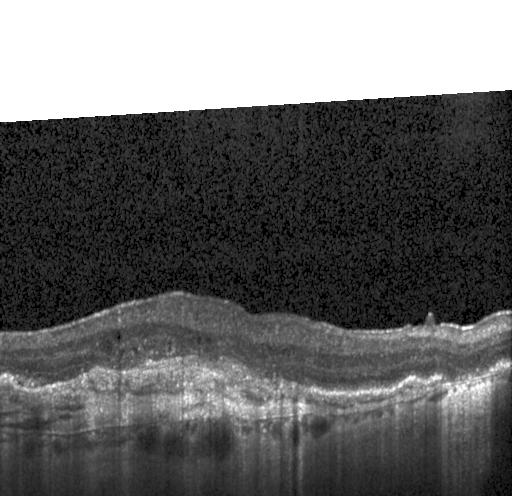 Optical coherence tomography scan, centered on the fovea, instrument: Heidelberg Spectralis, spectral-domain optical coherence tomography — Impression: choroidal neovascularization (CNV).